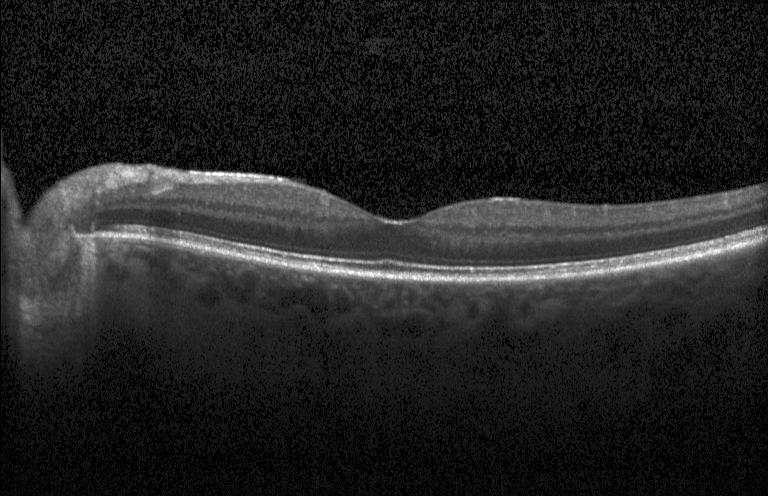

Dx: no choroidal neovascularization, diabetic macular edema, or drusen.